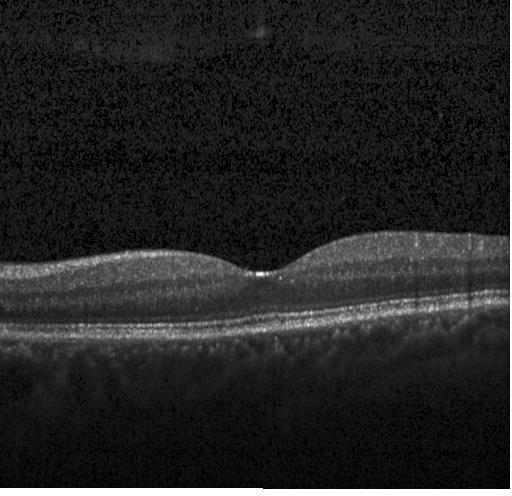 Macular OCT demonstrating no evidence of choroidal neovascularization, diabetic macular edema, or drusen.